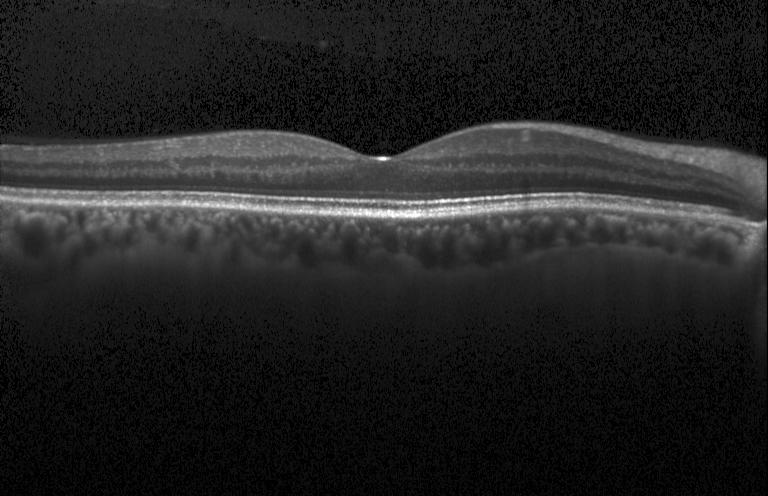
Spectral-domain OCT B-scan: no evidence of CNV, DME, or drusen.